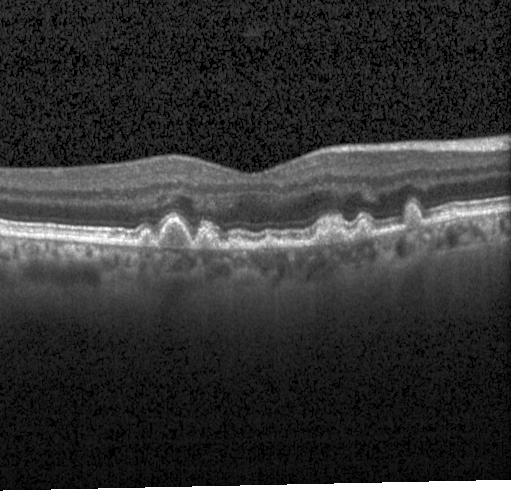
Retinal OCT B-scan.
This B-scan demonstrates sub-RPE drusenoid deposits.